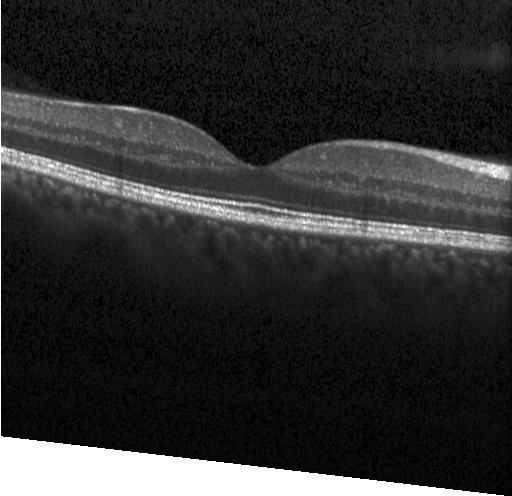
Optical coherence tomography scan, Heidelberg Spectralis OCT system, horizontal scan through the fovea. The scan shows no CNV, DME, or drusen.